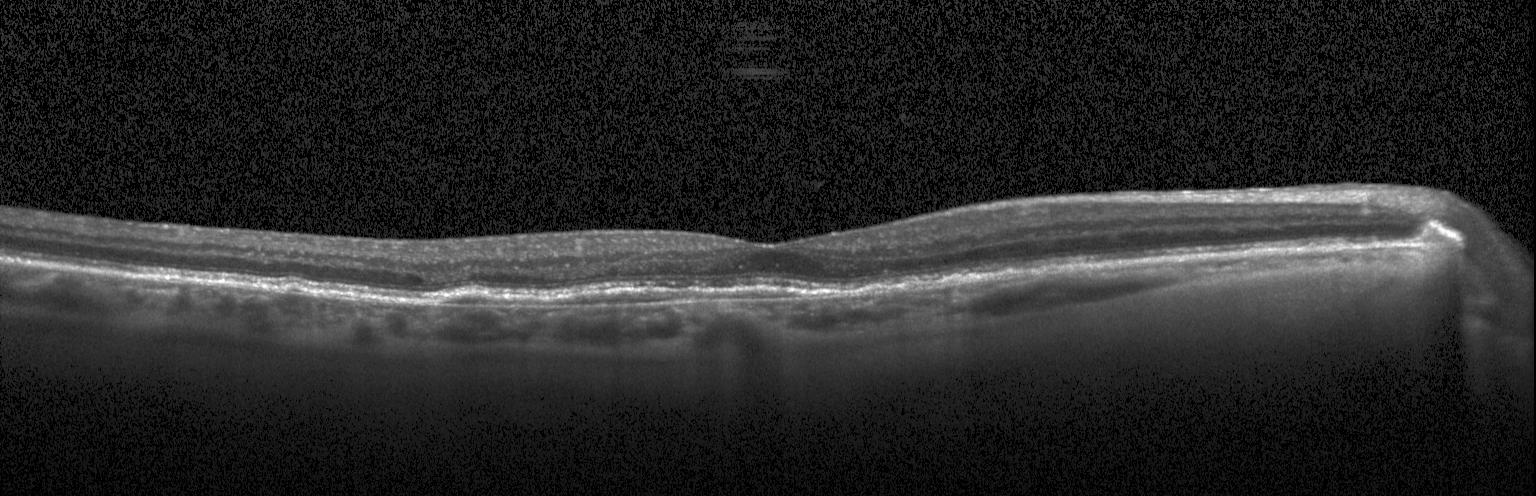 Optical coherence tomography scan
This B-scan demonstrates choroidal neovascularization (CNV).